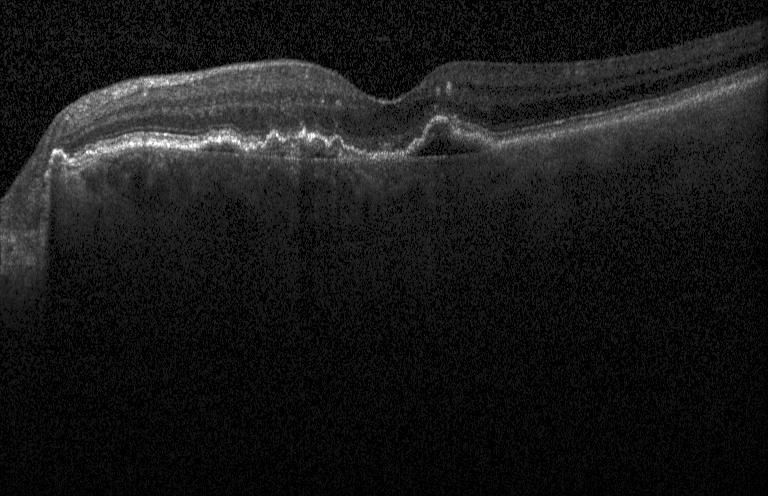 Spectral-domain OCT · through the macula · OCT B-scan.
Impression: choroidal neovascularization (CNV).